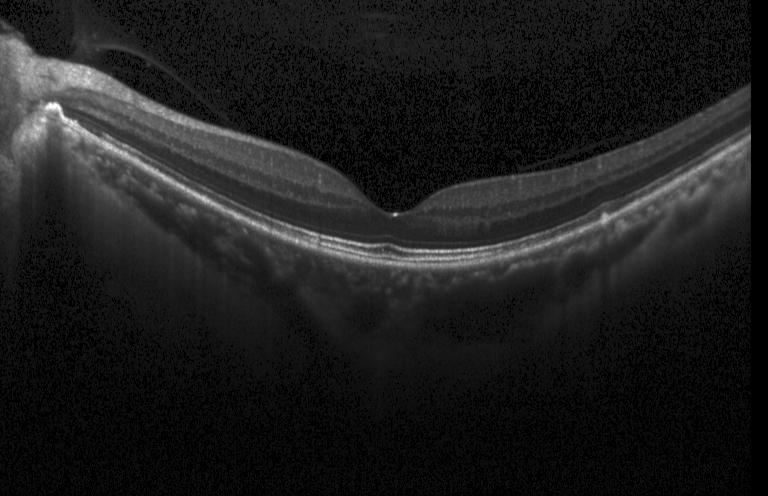
Diagnosis: sub-RPE drusenoid deposits.